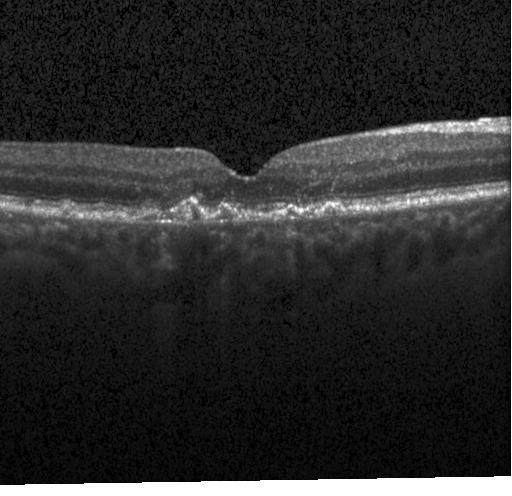 SD-OCT, macular scan, retinal OCT B-scan, instrument: Heidelberg Spectralis. A choroidal neovascular membrane.